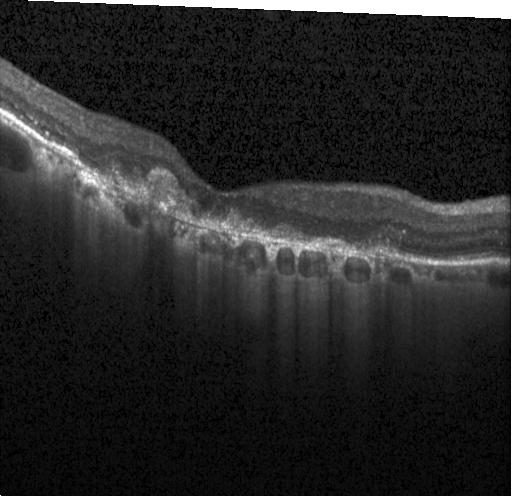

Macular OCT: a choroidal neovascular membrane.